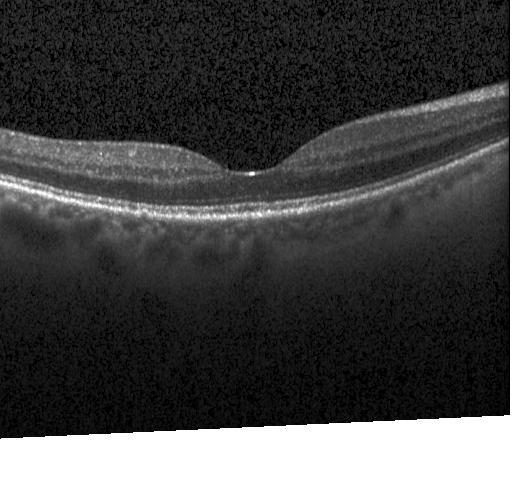 Diagnosis: no evidence of CNV, DME, or drusen.